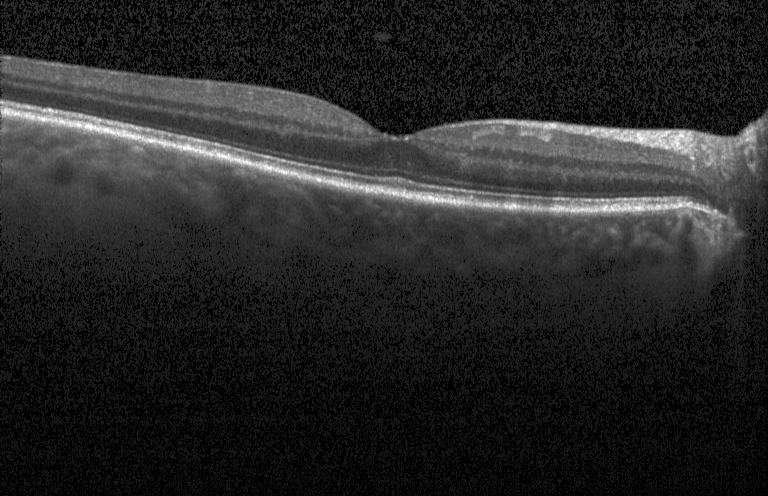
Through the macula · spectral-domain optical coherence tomography · optical coherence tomography scan — This B-scan demonstrates no CNV, no DME, and no drusen.